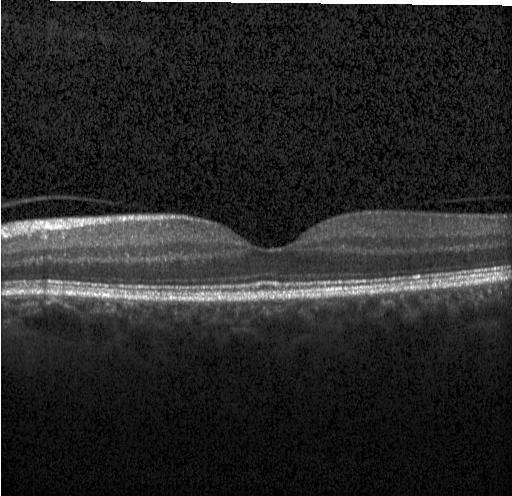

Assessment: no evidence of choroidal neovascularization, diabetic macular edema, or drusen.